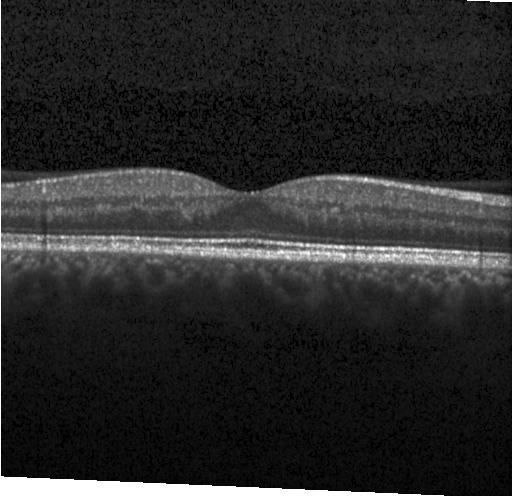 Heidelberg Spectralis · OCT line scan.
Macular OCT: neither CNV, DME, nor drusen.